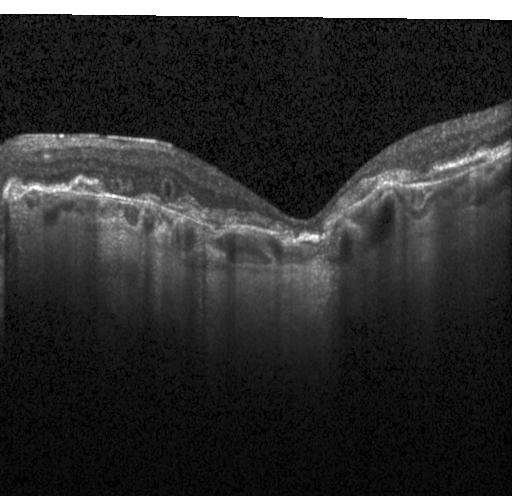 OCT B-scan — This B-scan demonstrates a choroidal neovascular membrane.